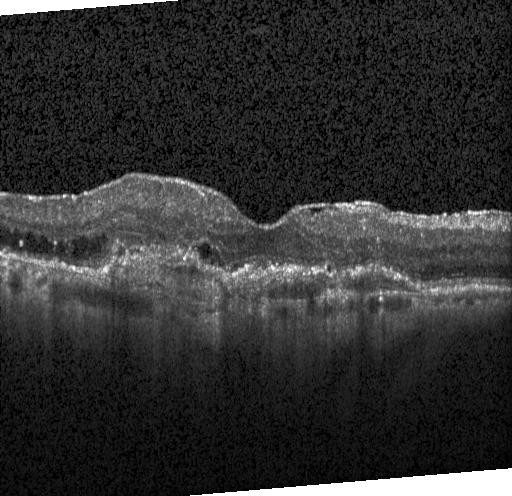
Retinal OCT B-scan. Horizontal scan through the fovea — Finding: a choroidal neovascular membrane.